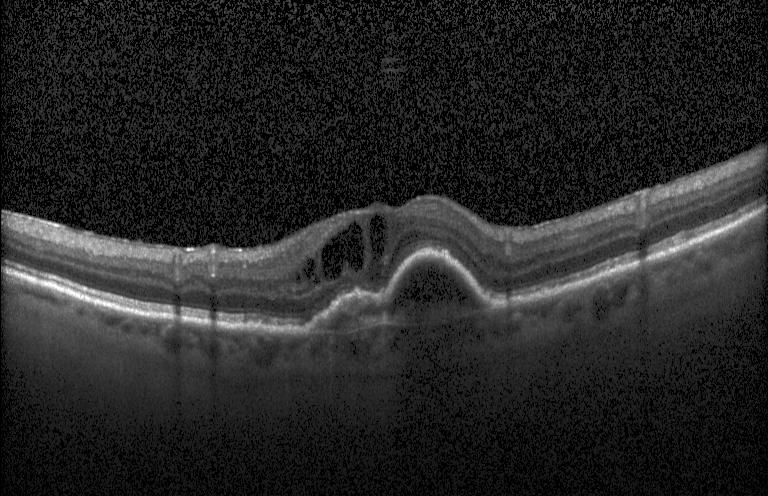
OCT B-scan. Impression: choroidal neovascularization (CNV).